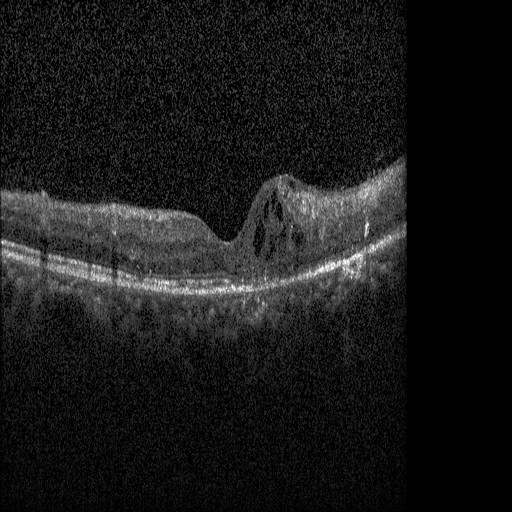 Impression: diabetic macular edema.